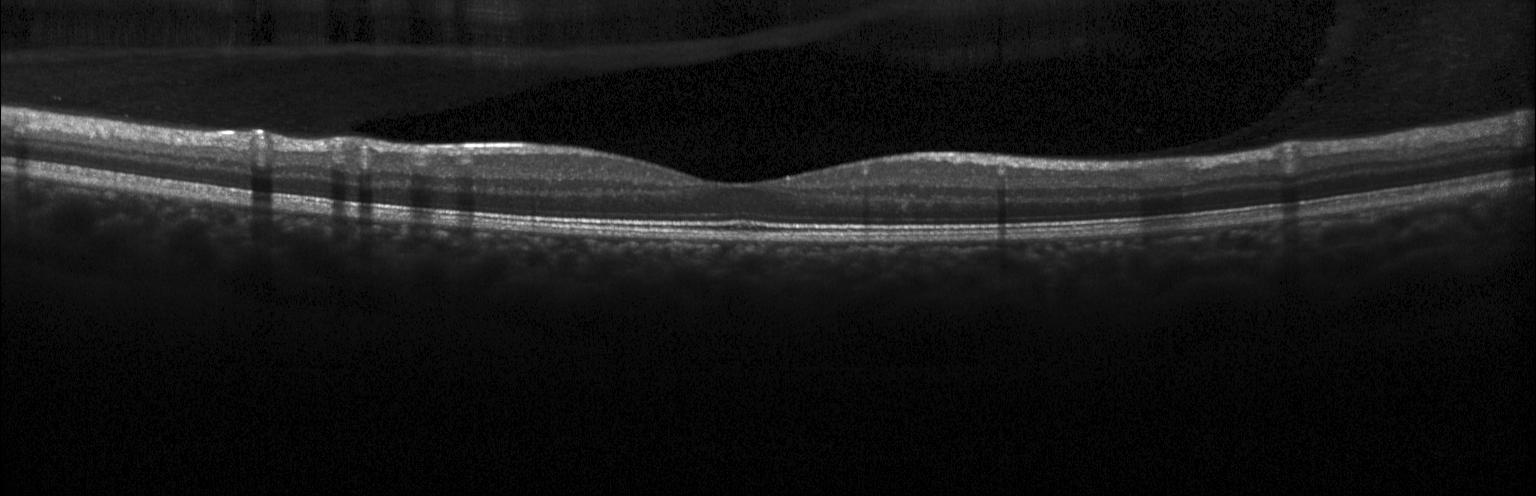
Horizontal scan through the fovea, retinal OCT cross-section. Neither CNV, DME, nor drusen.